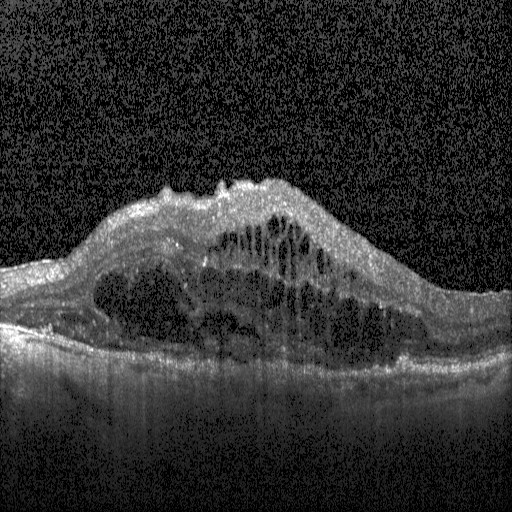

Finding: diabetic macular edema (DME).